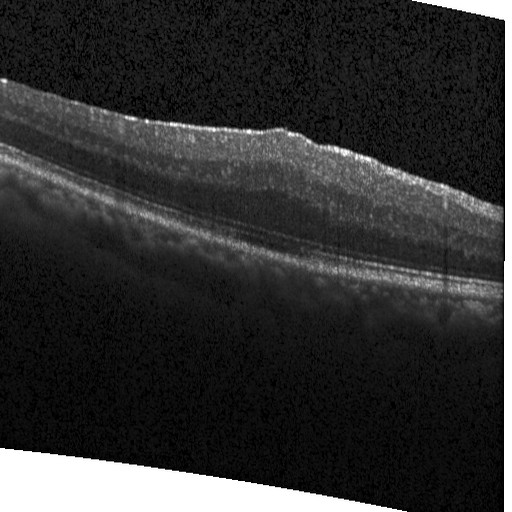

Diagnosis: DME.